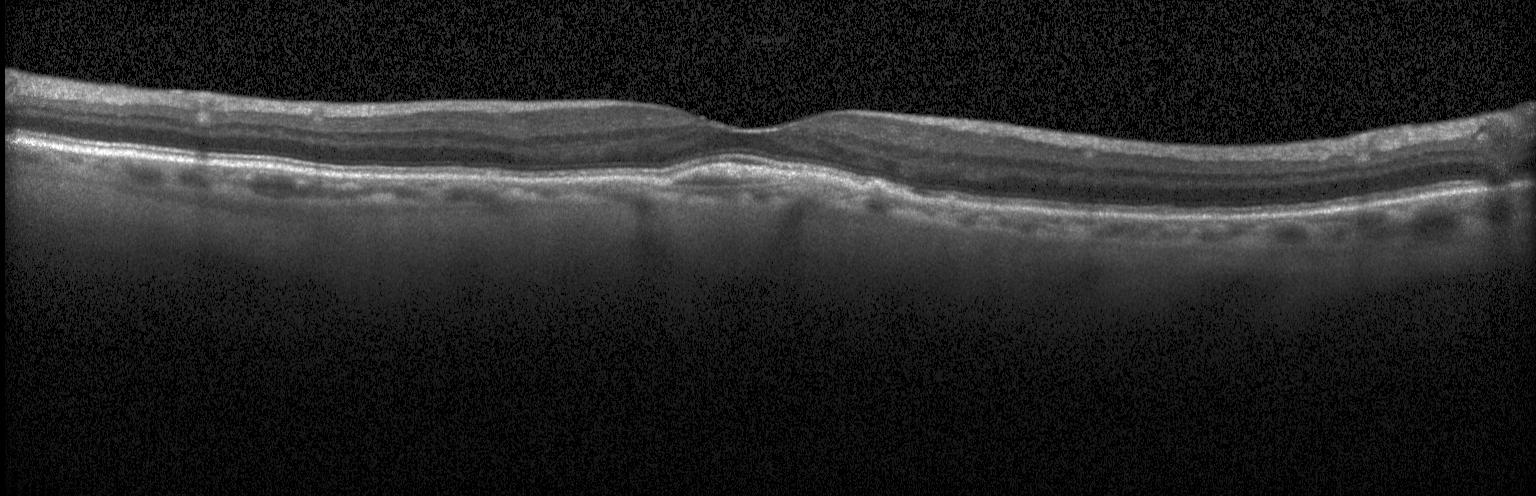
OCT B-scan showing choroidal neovascularization.